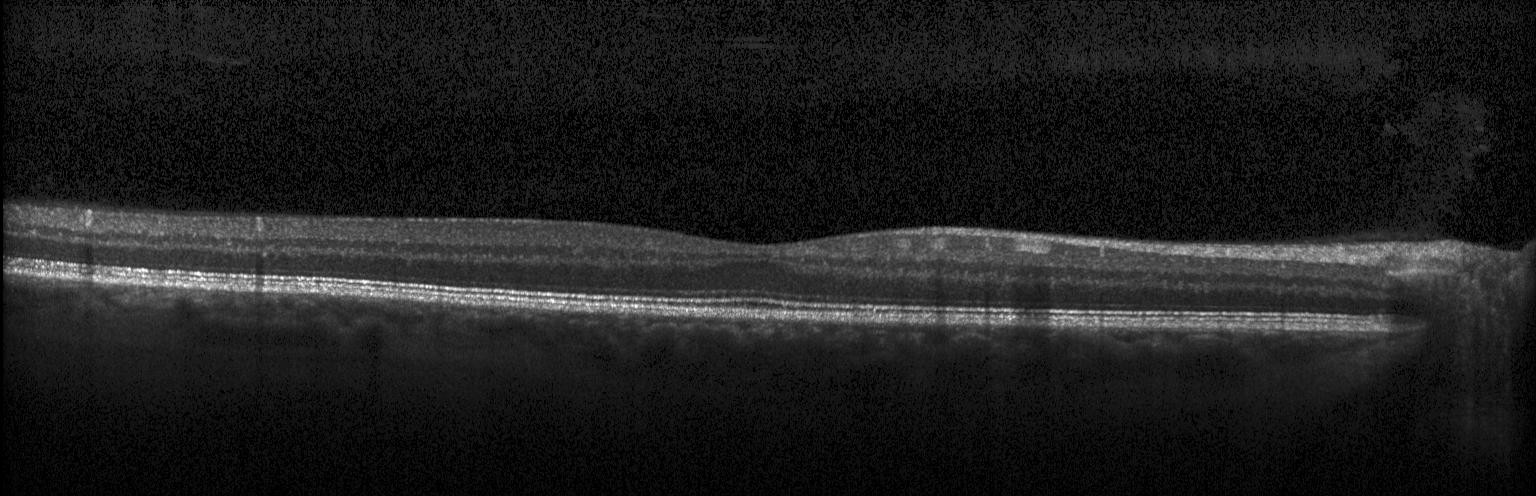 Heidelberg Spectralis OCT system; horizontal scan through the fovea; OCT line scan; spectral-domain optical coherence tomography. Macular OCT: neither choroidal neovascularization, diabetic macular edema, nor drusen.